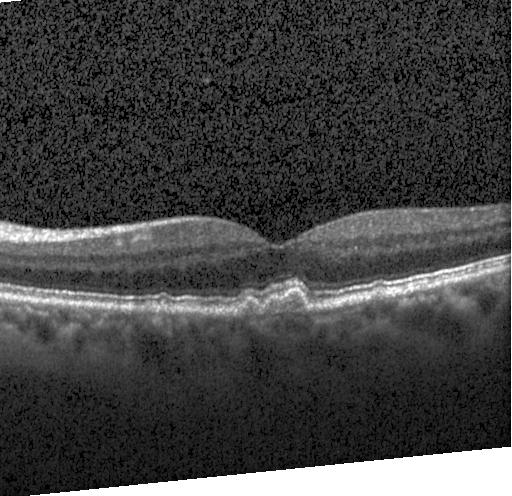

Optical coherence tomography scan · spectral-domain optical coherence tomography. Assessment: multiple drusen.